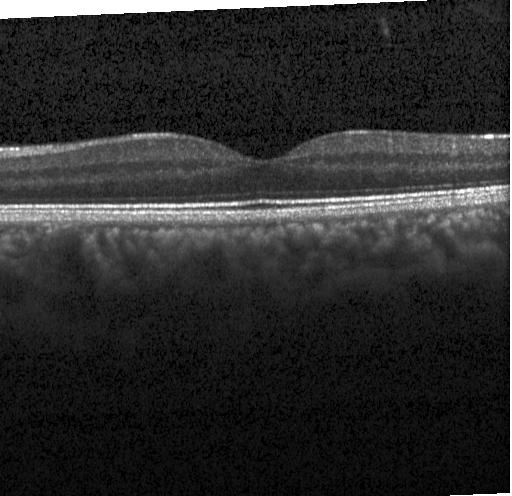

Heidelberg Spectralis; through the macula; retinal OCT cross-section; spectral-domain optical coherence tomography.
Impression: no choroidal neovascularization, no diabetic macular edema, and no drusen.